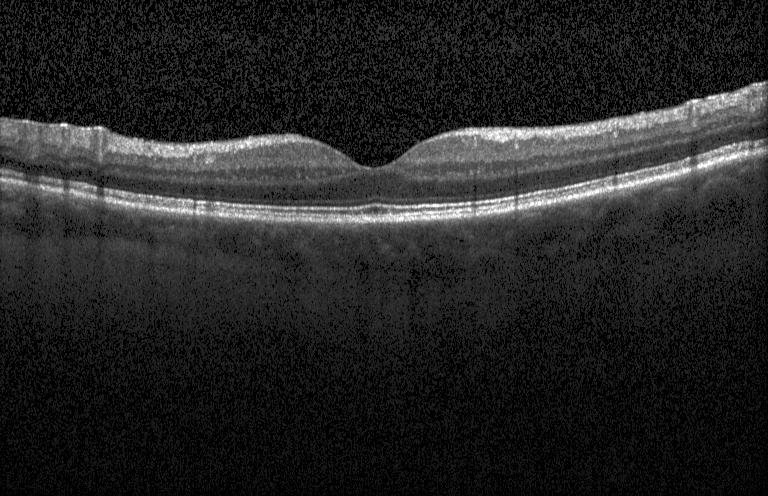

The scan shows neither choroidal neovascularization, diabetic macular edema, nor drusen.